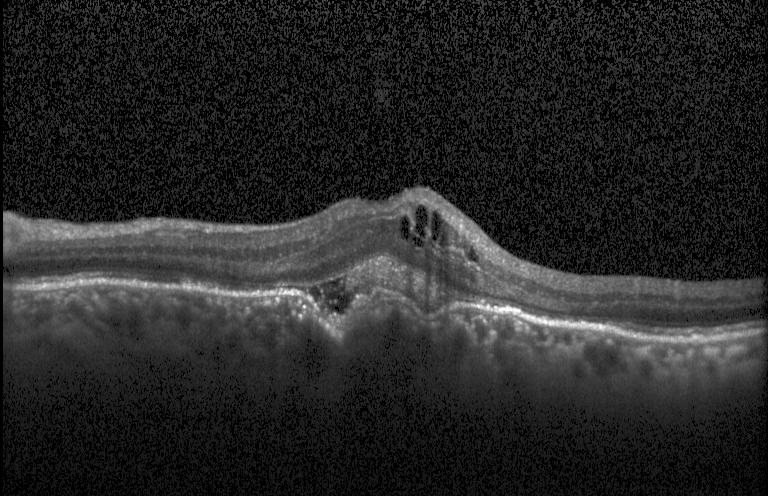
Fovea-centered; SD-OCT; Heidelberg Spectralis; optical coherence tomography scan — The scan shows CNV.